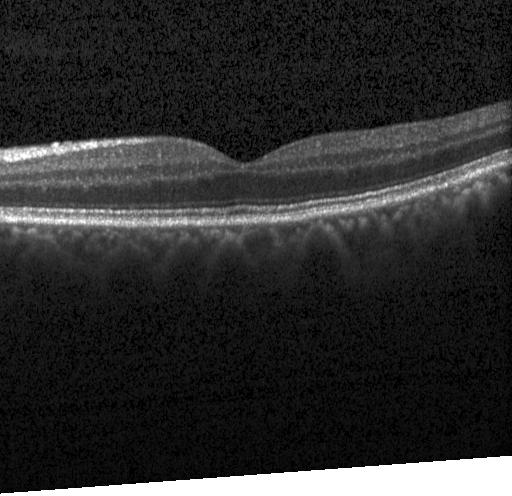
SD-OCT; optical coherence tomography B-scan — Finding: no evidence of CNV, DME, or drusen.